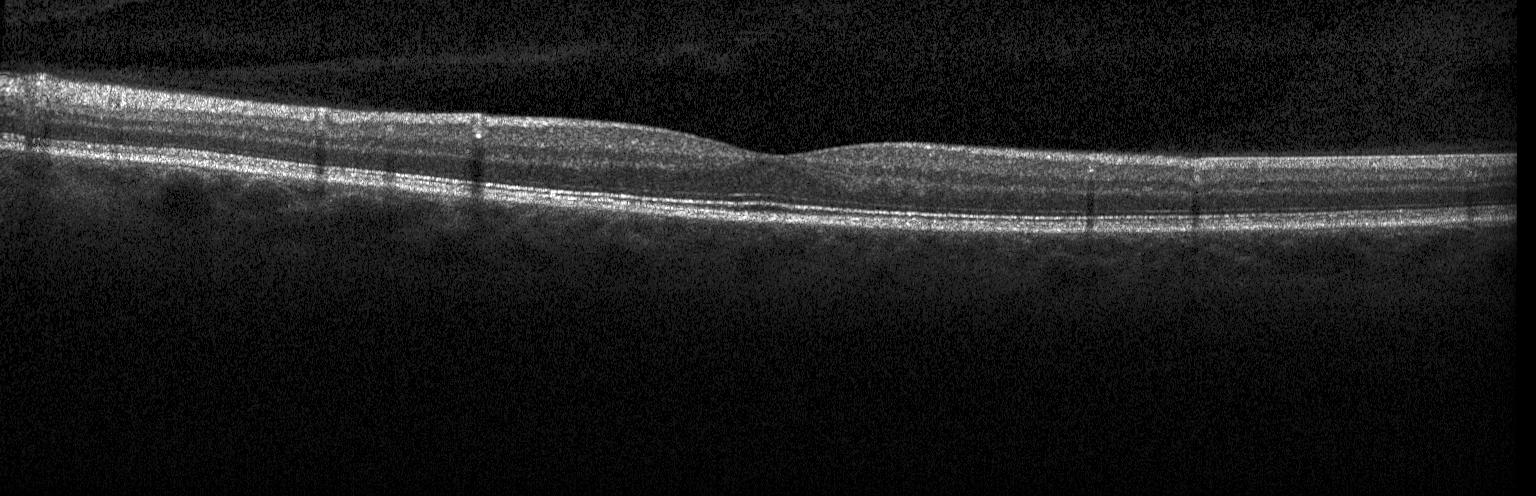
Through the macula; instrument: Heidelberg Spectralis; OCT line scan; spectral-domain OCT
This B-scan demonstrates no choroidal neovascularization, no diabetic macular edema, and no drusen.